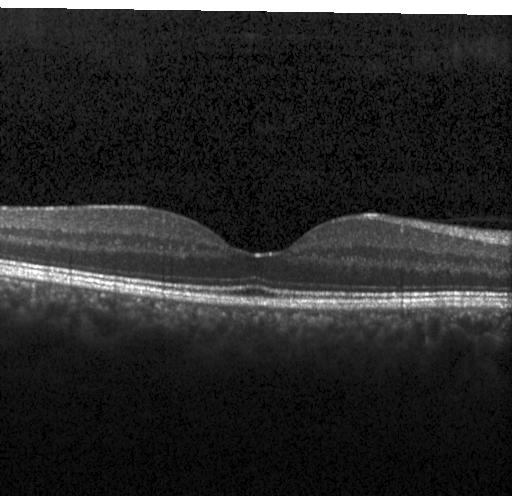 Optical coherence tomography B-scan, through the macula. Impression: no choroidal neovascularization, diabetic macular edema, or drusen.